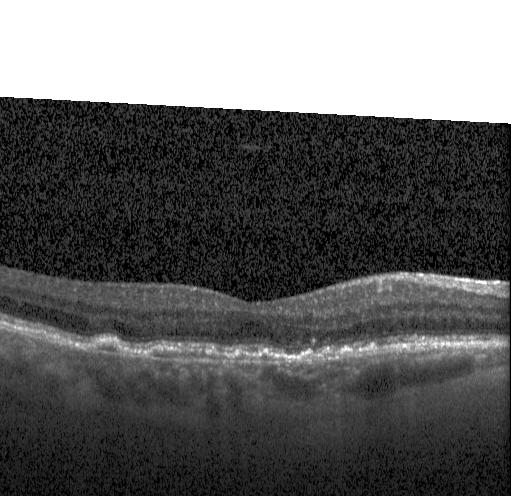 Optical coherence tomography B-scan. Heidelberg Spectralis OCT system
Assessment: a choroidal neovascular membrane.